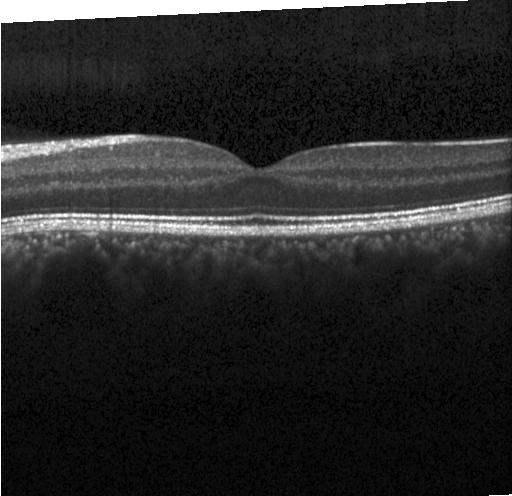
Through the macula · optical coherence tomography scan — Impression: no CNV, no DME, and no drusen.